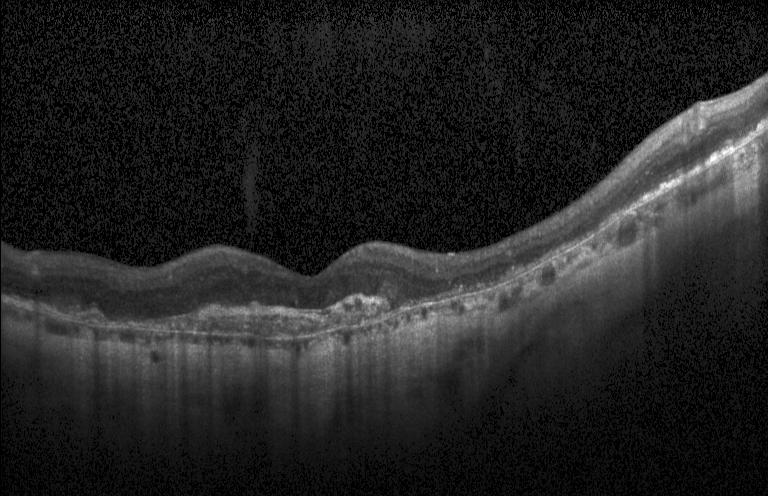
Fovea-centered · OCT B-scan.
Finding: choroidal neovascularization (CNV).